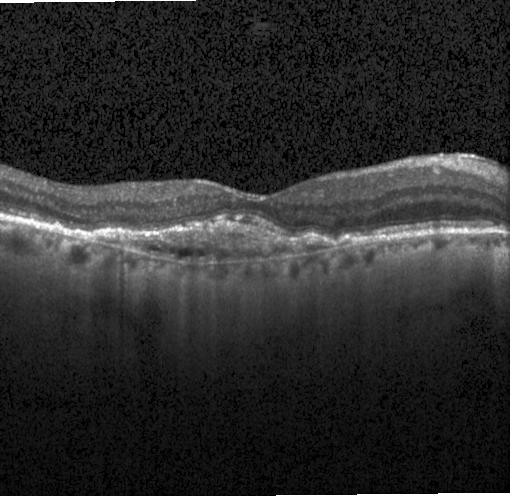
Through the macula. Spectral-domain OCT. OCT line scan. Heidelberg Spectralis OCT system
Assessment: a choroidal neovascular membrane.